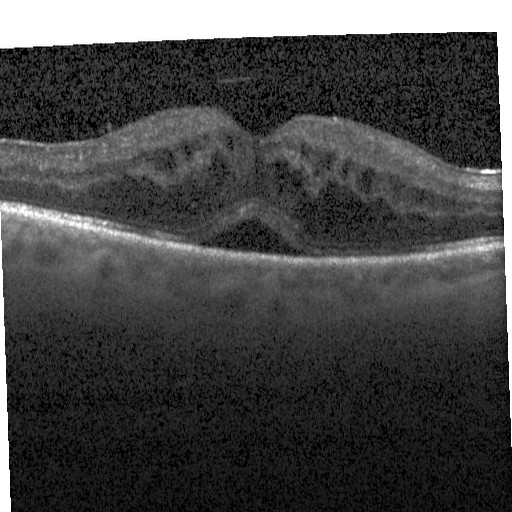

Macular OCT demonstrating DME.